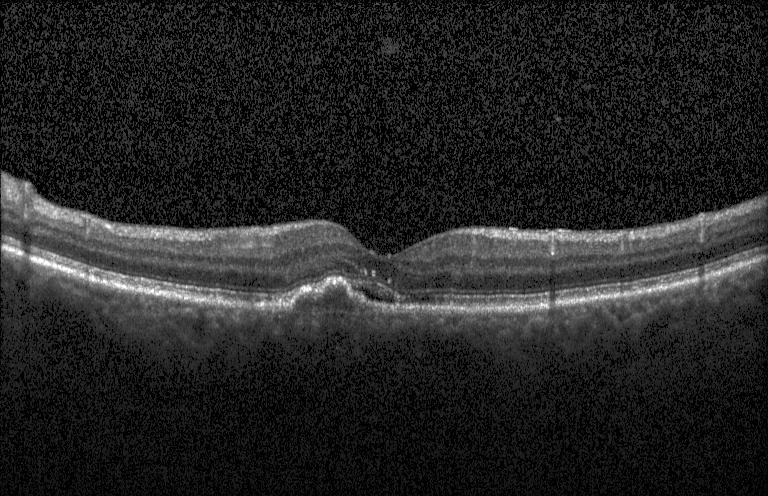 OCT line scan · through the macula. Finding: a choroidal neovascular membrane.